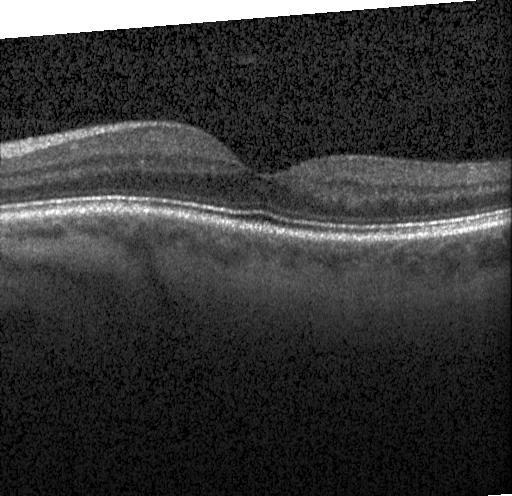

Spectral-domain OCT B-scan: neither choroidal neovascularization, diabetic macular edema, nor drusen.